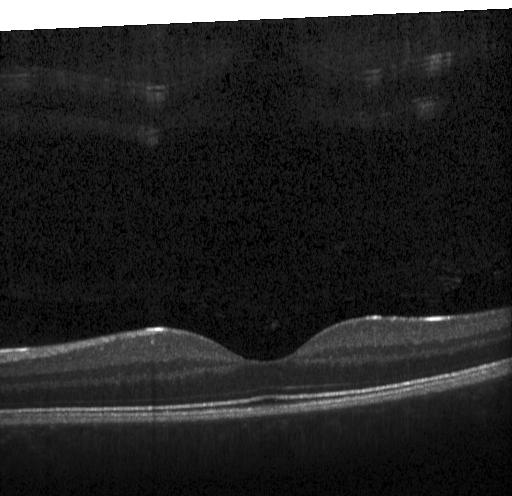
Acquired on a Heidelberg Spectralis. Optical coherence tomography B-scan. Spectral-domain optical coherence tomography
Dx: neither choroidal neovascularization, diabetic macular edema, nor drusen.